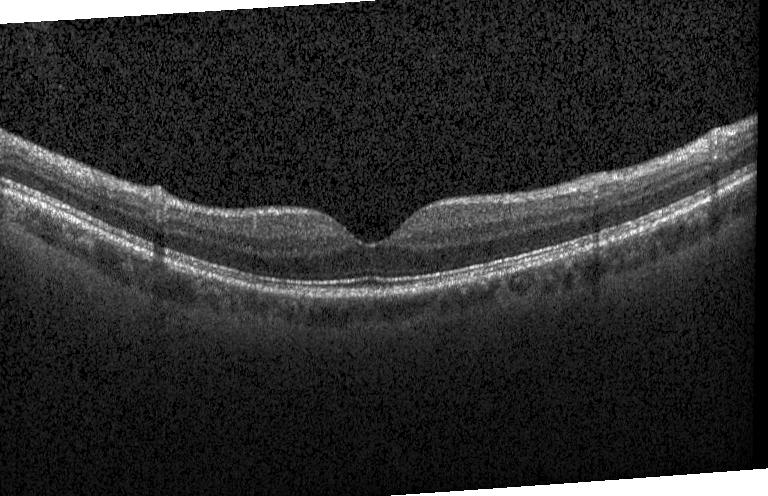

Spectral-domain OCT B-scan: no choroidal neovascularization, no diabetic macular edema, and no drusen.